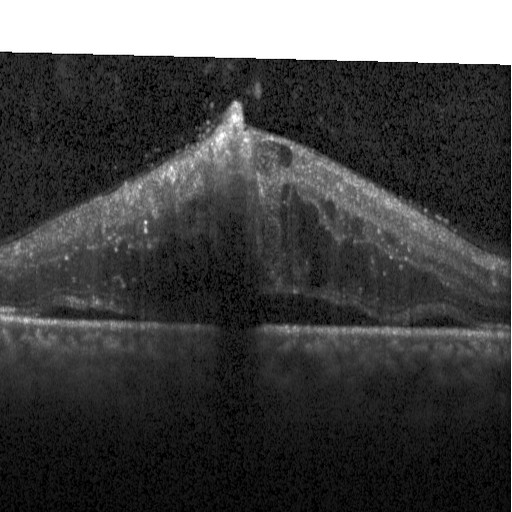 Diagnosis: diabetic macular edema.